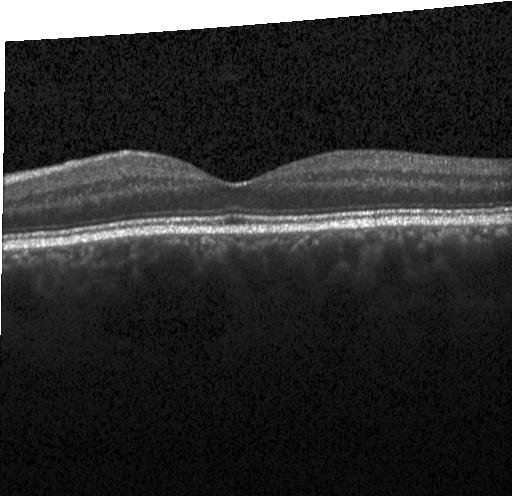
Through the macula. Spectral-domain OCT. OCT line scan. Acquired on a Heidelberg Spectralis
The scan shows no choroidal neovascularization, diabetic macular edema, or drusen.